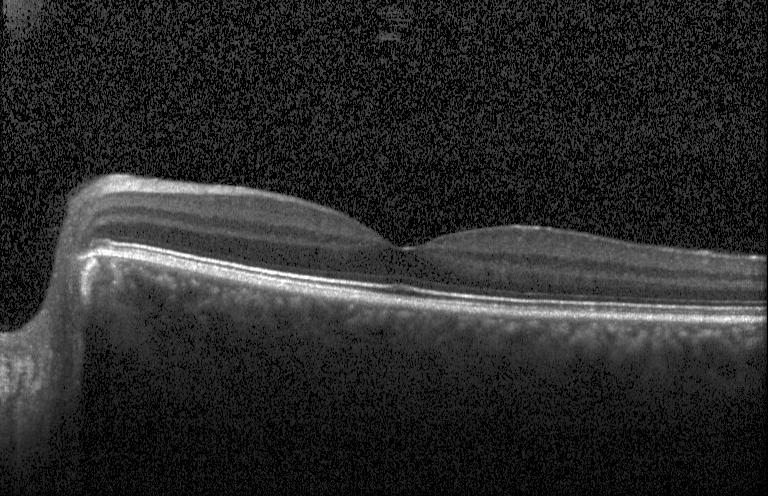
Retinal OCT B-scan — OCT finding: no choroidal neovascularization, no diabetic macular edema, and no drusen.